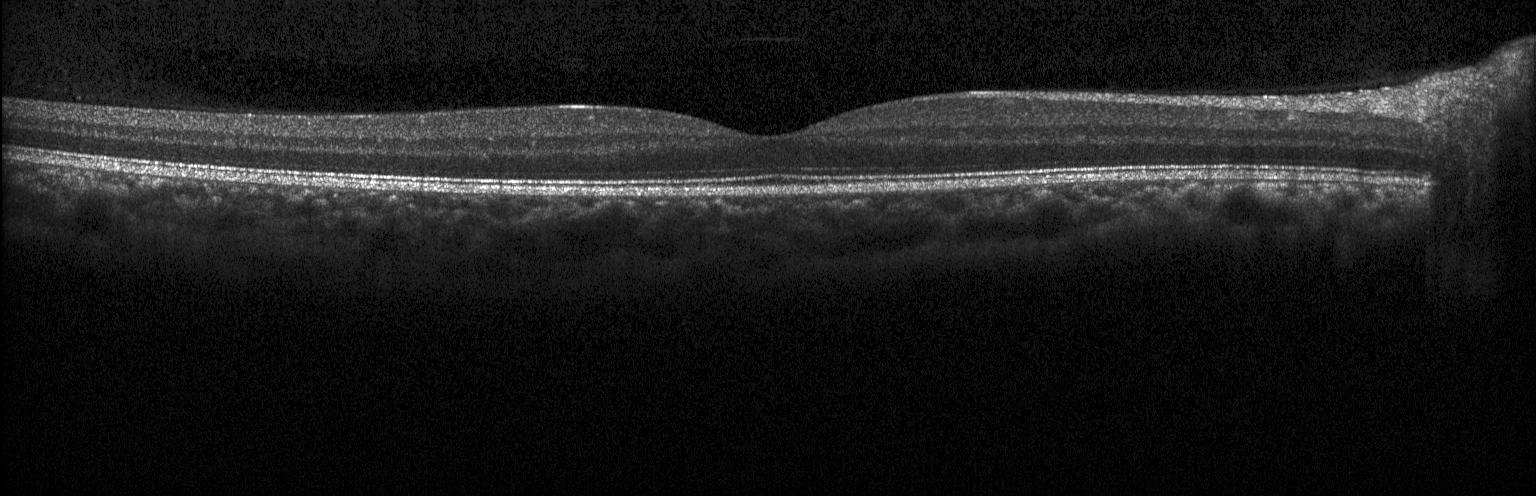

Assessment: no CNV, DME, or drusen.